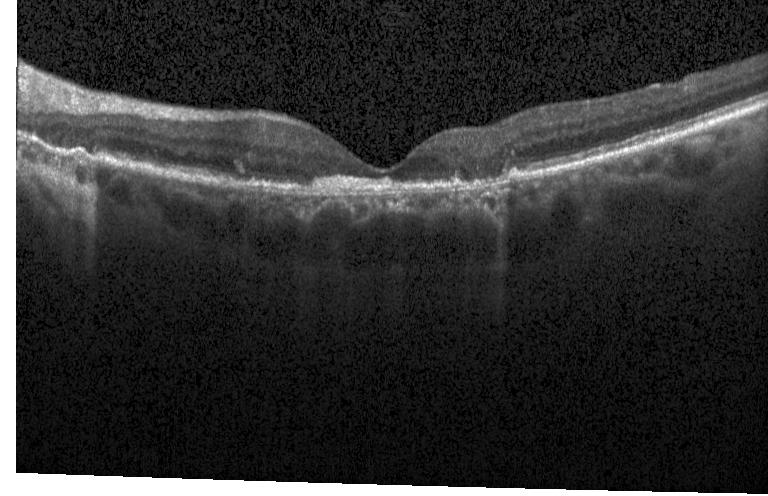

OCT line scan.
Assessment: CNV.